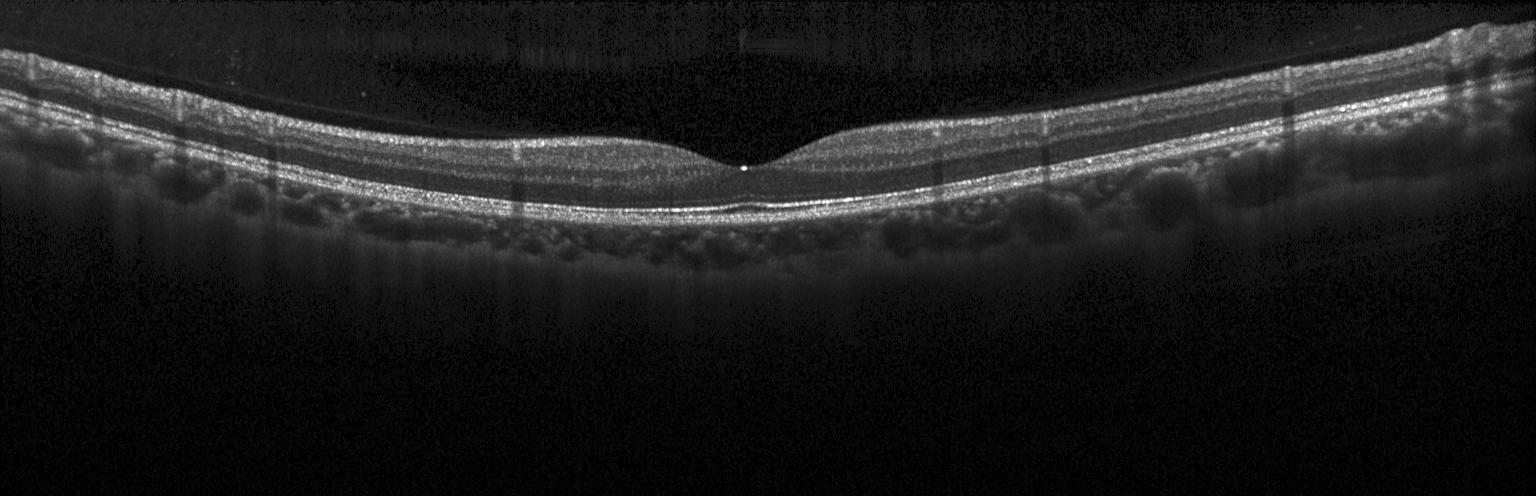
Macular OCT: no choroidal neovascularization, no diabetic macular edema, and no drusen.